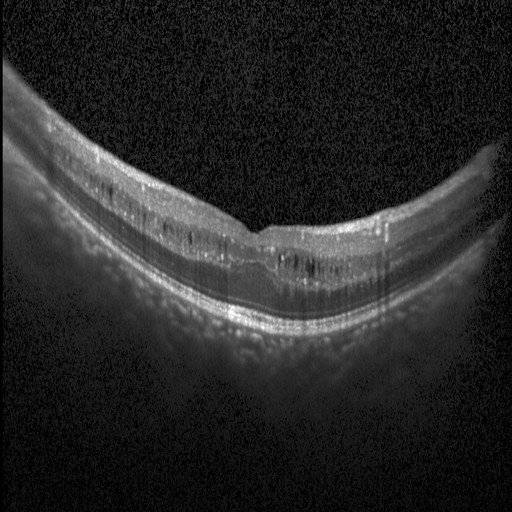

Optical coherence tomography B-scan · instrument: Heidelberg Spectralis · spectral-domain OCT.
Finding: diabetic macular edema (DME).